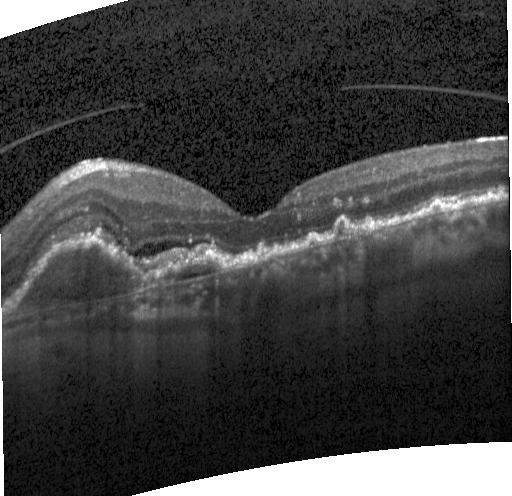

Macular OCT: choroidal neovascularization.